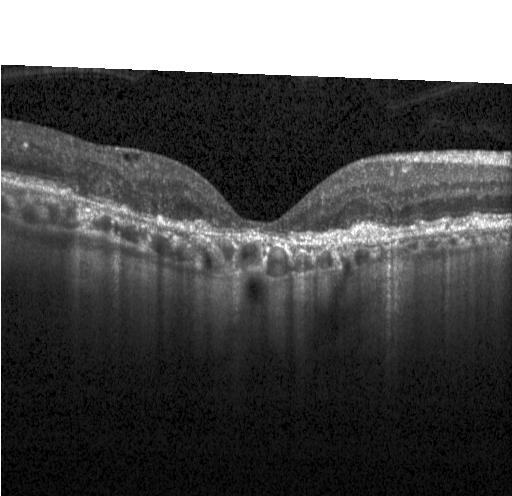

Retinal OCT cross-section · Heidelberg Spectralis · spectral-domain optical coherence tomography. Finding: a choroidal neovascular membrane.